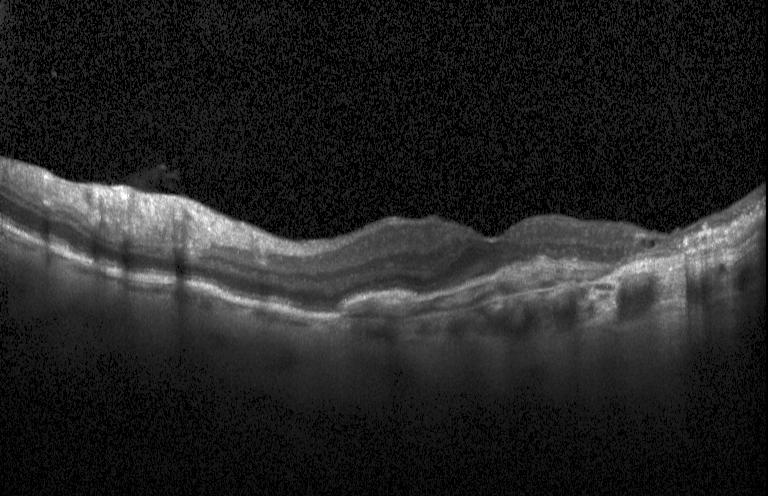 Retinal OCT B-scan · Heidelberg Spectralis OCT system · spectral-domain OCT · centered on the fovea.
Impression: CNV.